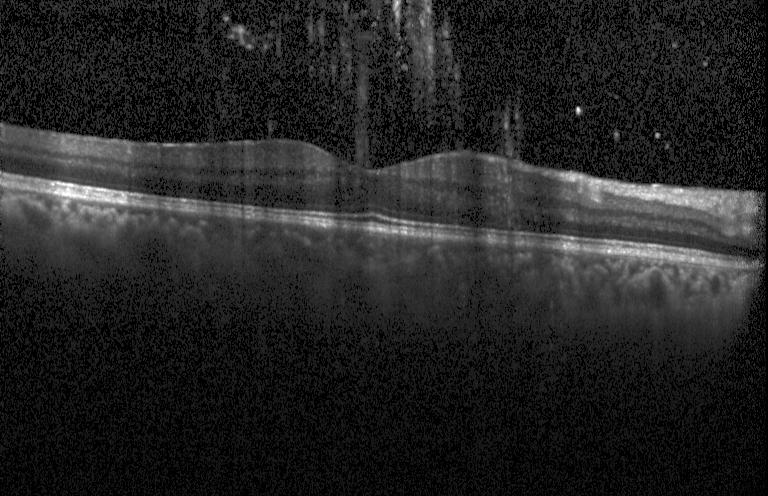

OCT scan showing no CNV, DME, or drusen.